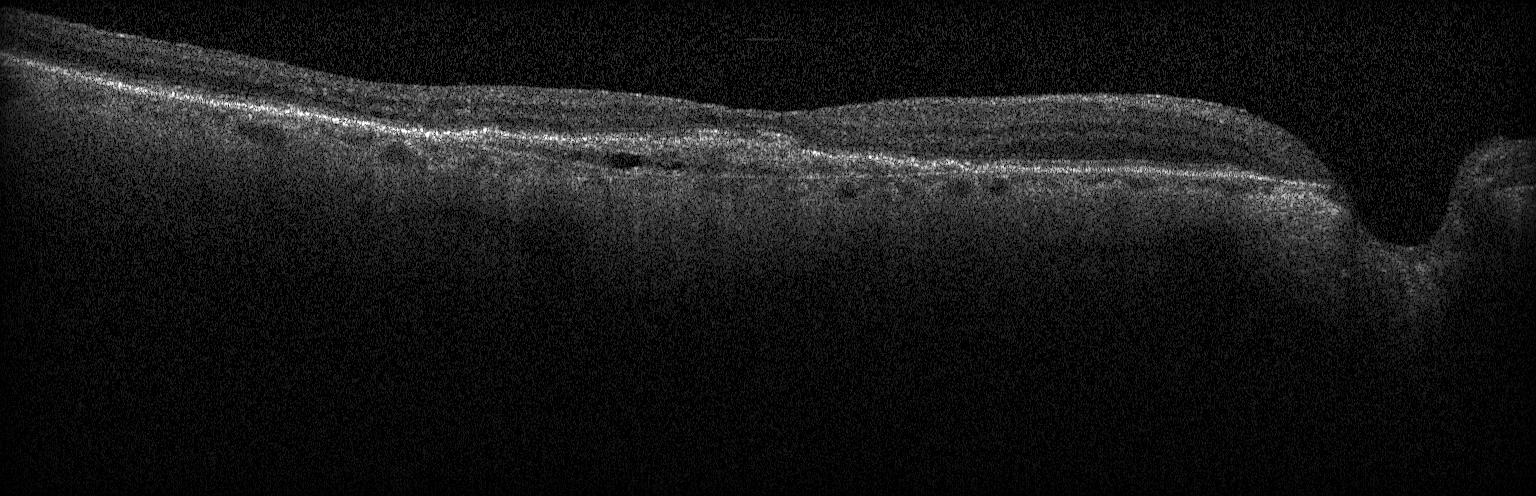
Retinal OCT B-scan — Impression: CNV.